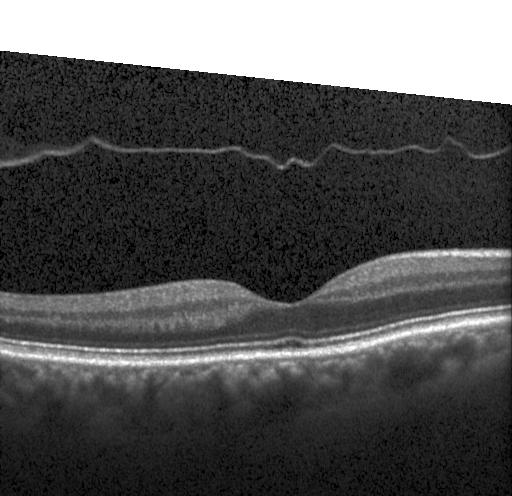

OCT finding: no evidence of choroidal neovascularization, diabetic macular edema, or drusen.